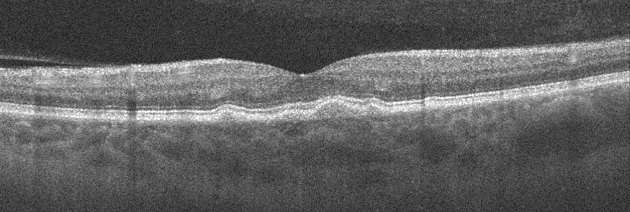
Oculus sinister; retinal OCT cross-section. Impression: AMD.